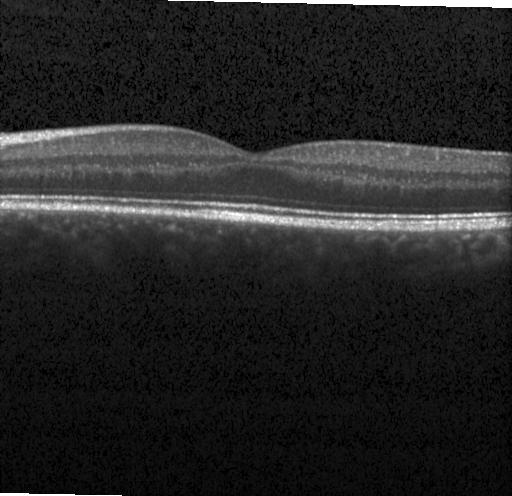 The scan shows no CNV, DME, or drusen.